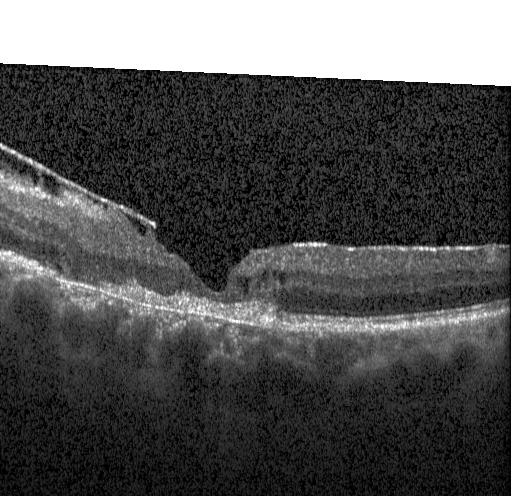 Retinal OCT B-scan. Spectral-domain optical coherence tomography — Finding: a choroidal neovascular membrane.